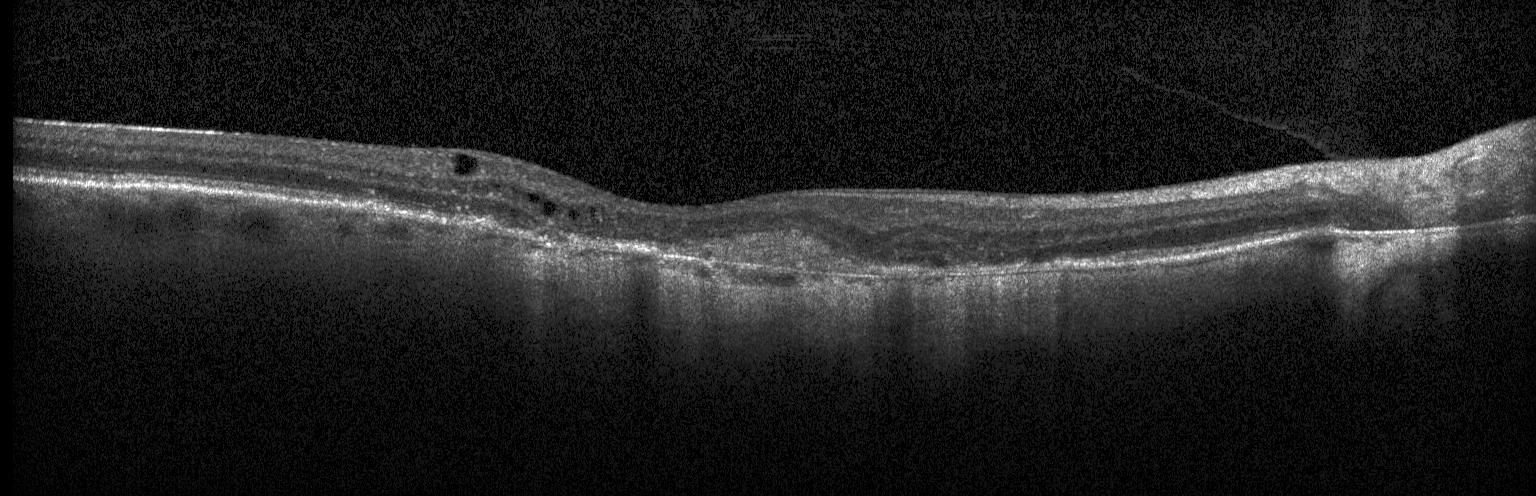

Acquired on a Heidelberg Spectralis. Retinal OCT B-scan. The scan shows choroidal neovascularization (CNV).